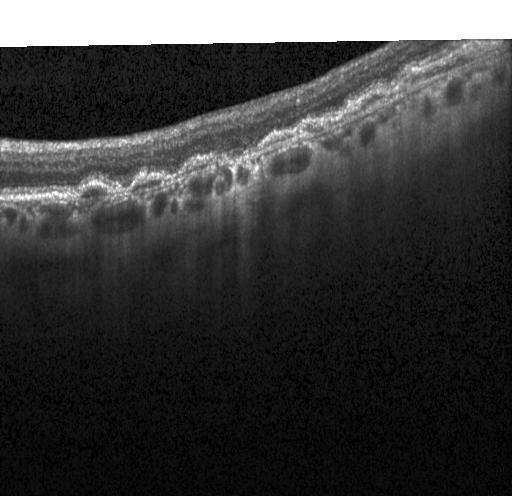

Diagnosis: choroidal neovascularization.